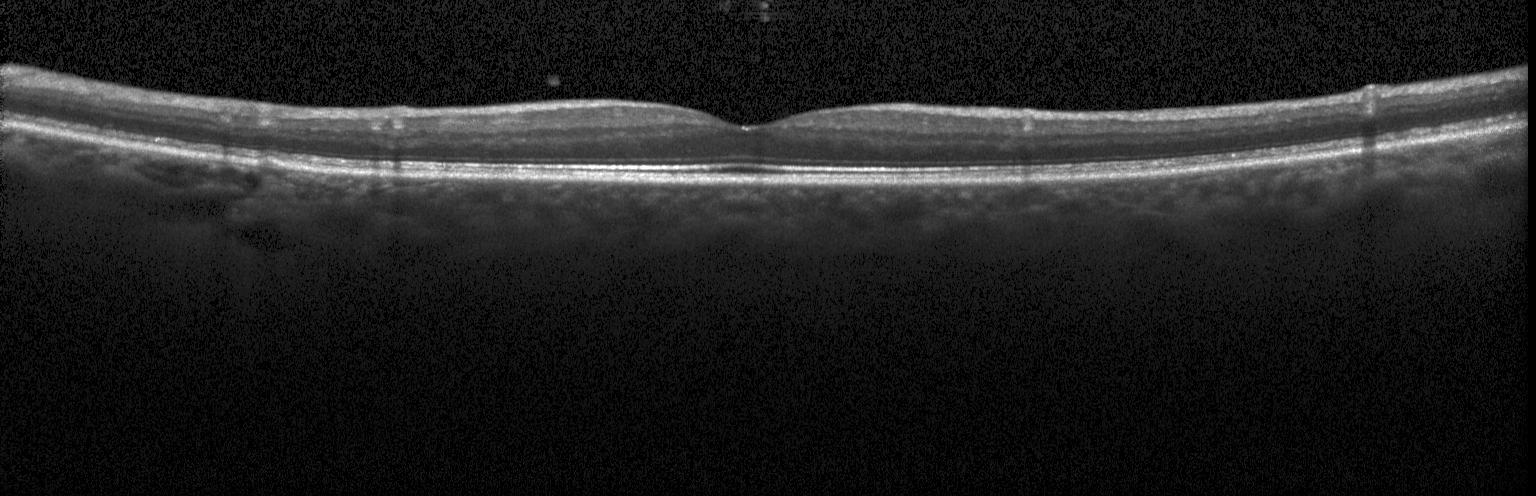

Horizontal scan through the fovea · spectral-domain optical coherence tomography · Heidelberg Spectralis OCT system · retinal OCT B-scan.
Impression: no CNV, DME, or drusen.